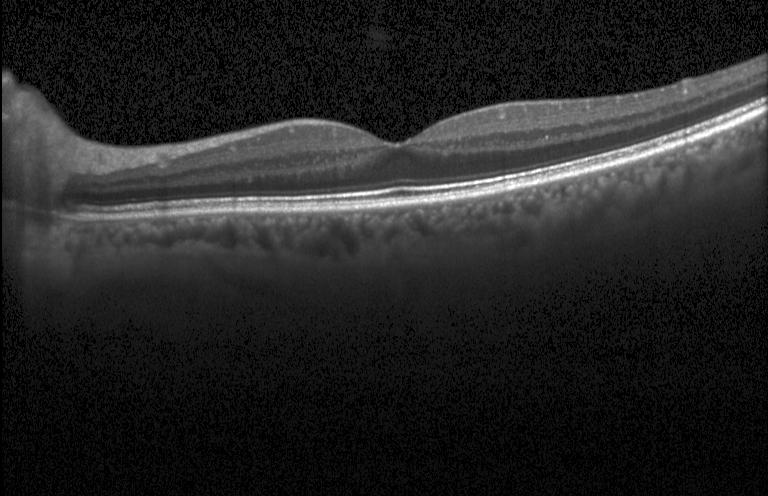 Dx: no choroidal neovascularization, no diabetic macular edema, and no drusen.